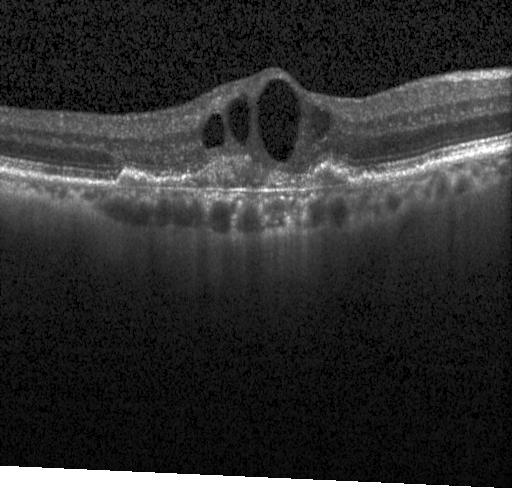
Through the macula · retinal OCT B-scan · Heidelberg Spectralis · spectral-domain OCT.
Impression: choroidal neovascularization (CNV).